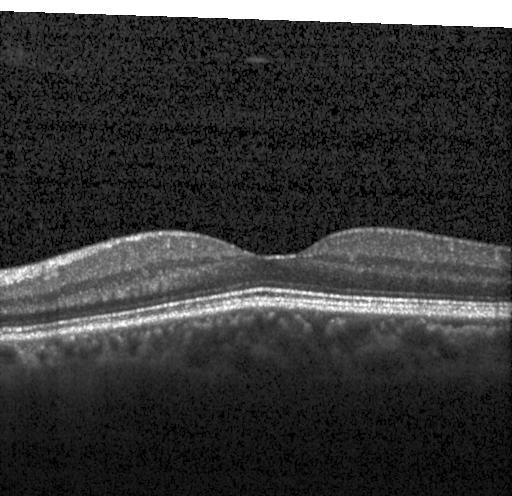
OCT line scan
Assessment: no evidence of CNV, DME, or drusen.